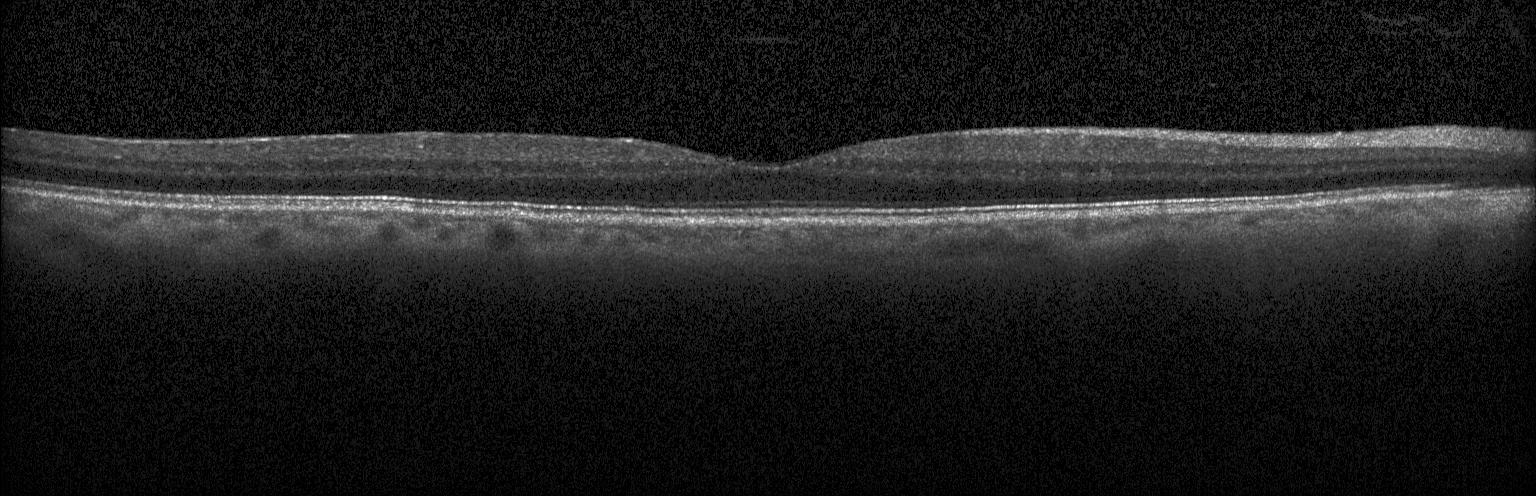

Diagnosis: no choroidal neovascularization, diabetic macular edema, or drusen.